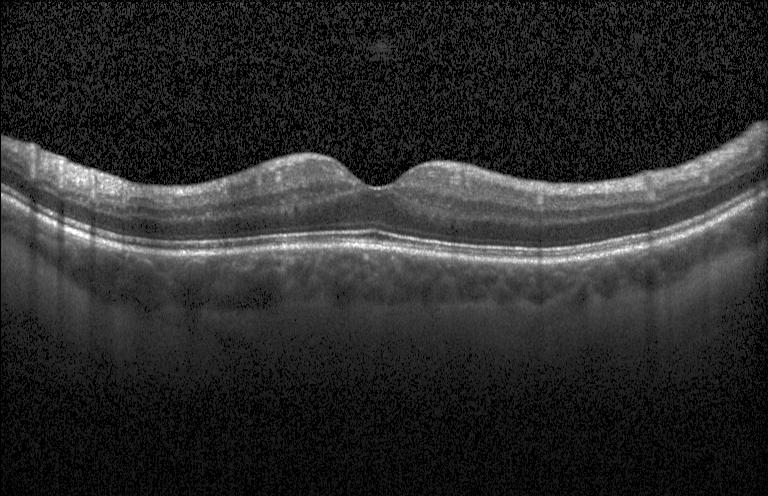

Optical coherence tomography B-scan. Spectral-domain OCT — Assessment: no CNV, DME, or drusen.